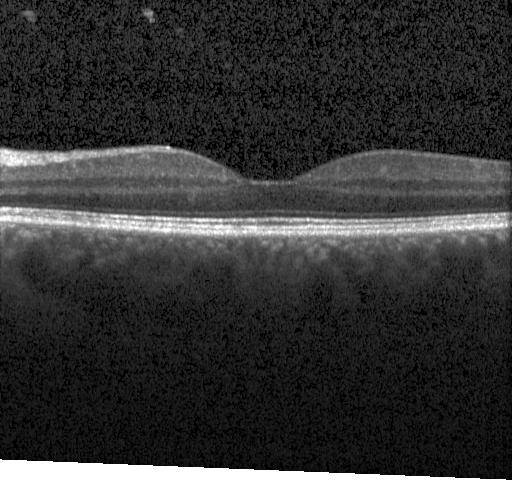

Optical coherence tomography B-scan; macular scan — Impression: no CNV, no DME, and no drusen.